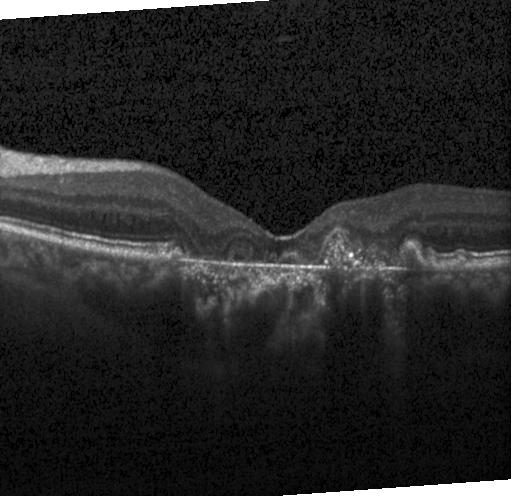 Assessment: choroidal neovascularization.